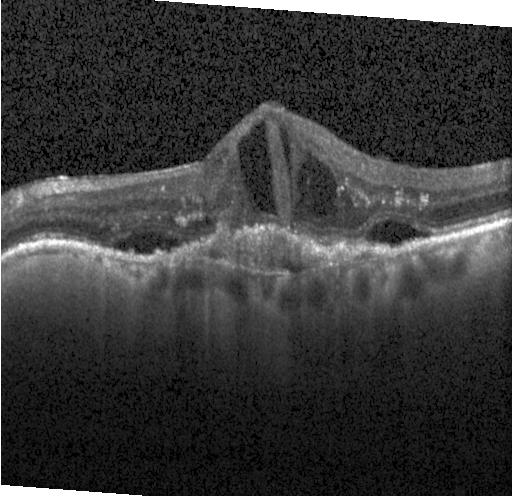

Macular OCT: choroidal neovascularization.